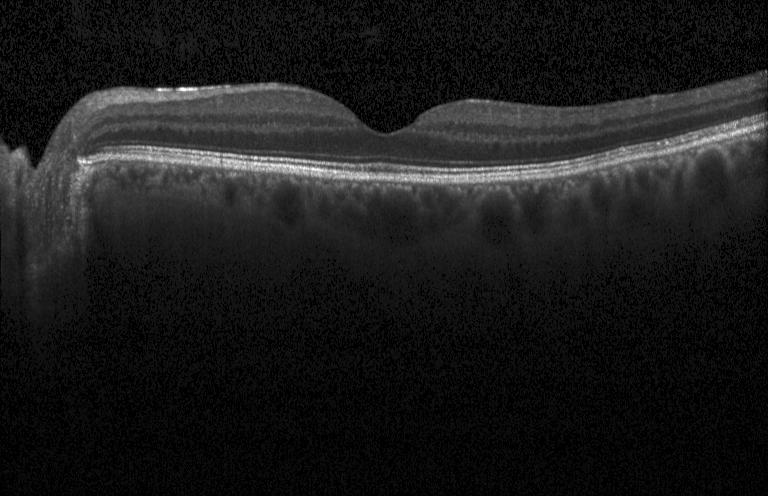 SD-OCT; Heidelberg Spectralis; fovea-centered; retinal OCT cross-section
Diagnosis: no CNV, no DME, and no drusen.